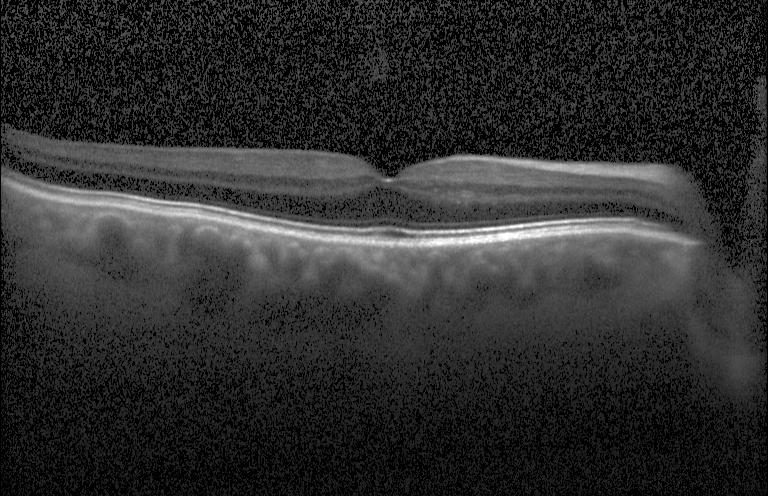

This B-scan demonstrates no CNV, no DME, and no drusen.